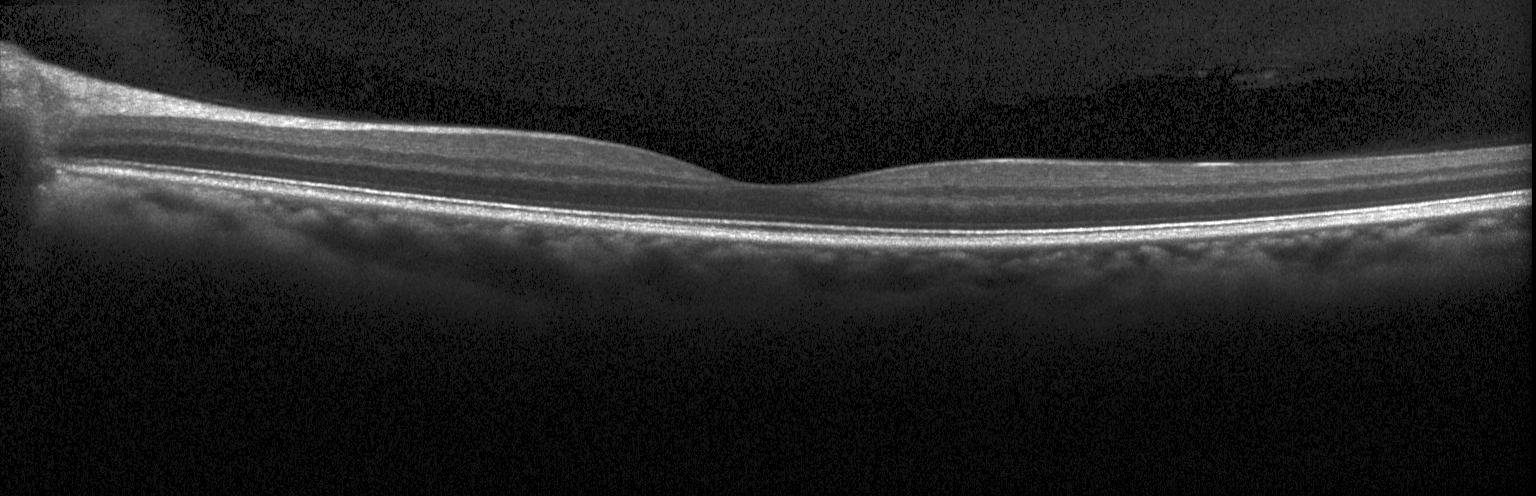 Finding: no evidence of choroidal neovascularization, diabetic macular edema, or drusen.